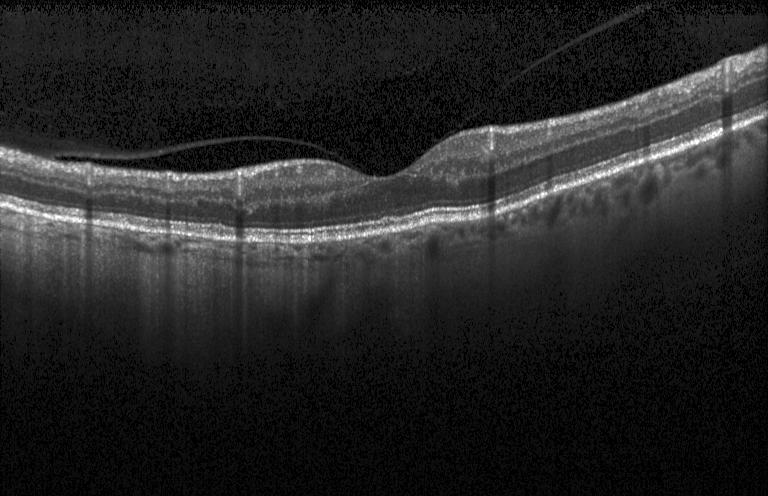 SD-OCT; retinal OCT cross-section
The scan shows no choroidal neovascularization, no diabetic macular edema, and no drusen.